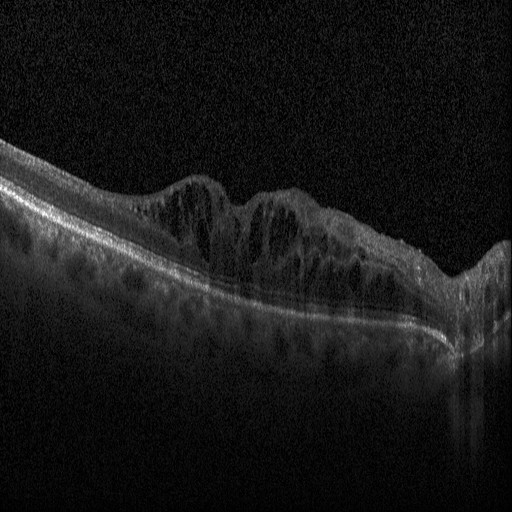 Dx: diabetic macular edema.